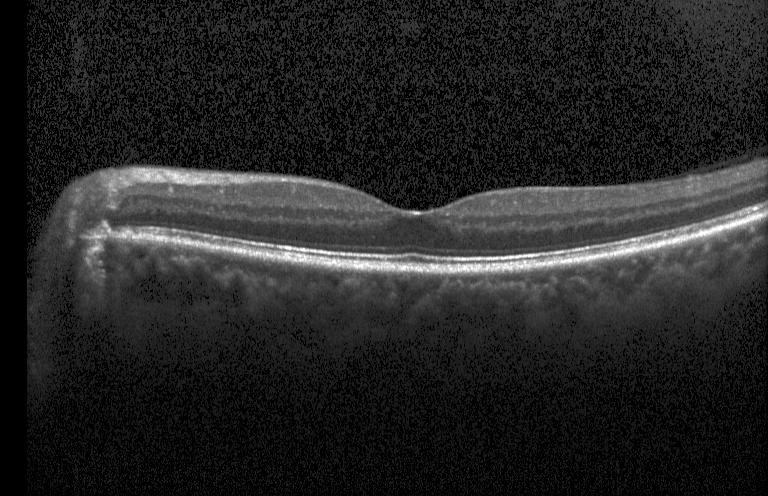
Assessment: no choroidal neovascularization, no diabetic macular edema, and no drusen.